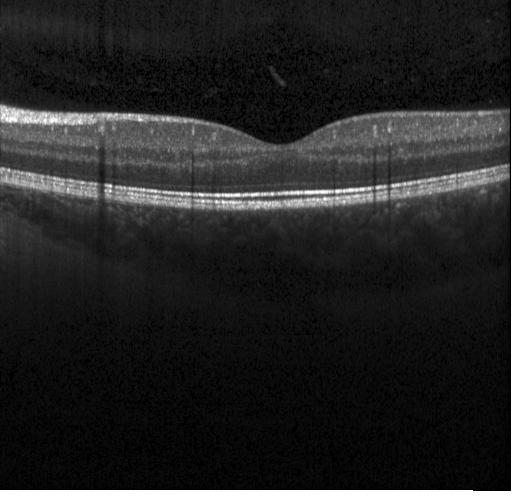
OCT scan showing no evidence of CNV, DME, or drusen.